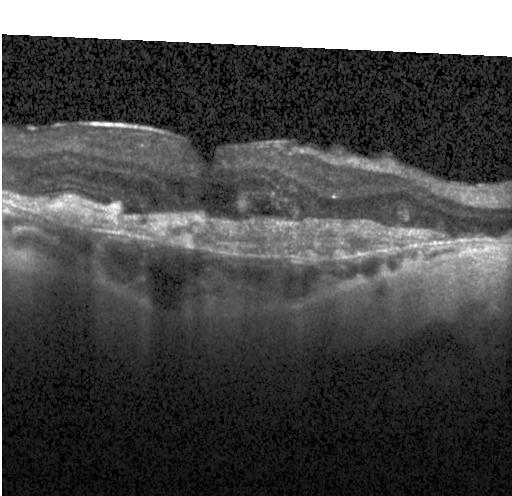
Retinal OCT B-scan.
Dx: a choroidal neovascular membrane.